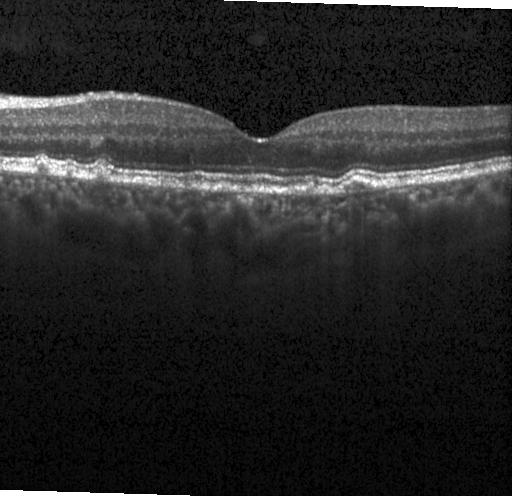

The scan shows drusen.